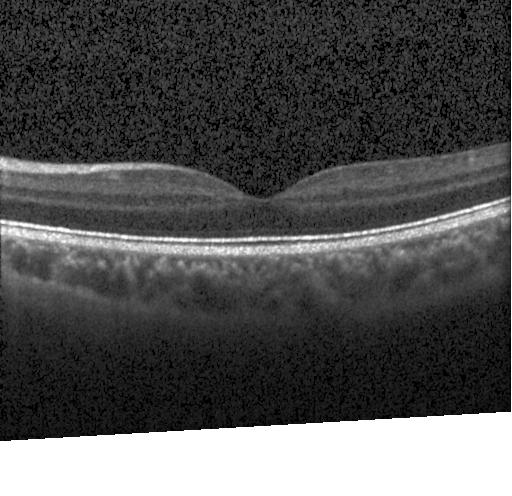 Through the macula; Heidelberg Spectralis; retinal OCT B-scan; SD-OCT. Diagnosis: no CNV, DME, or drusen.